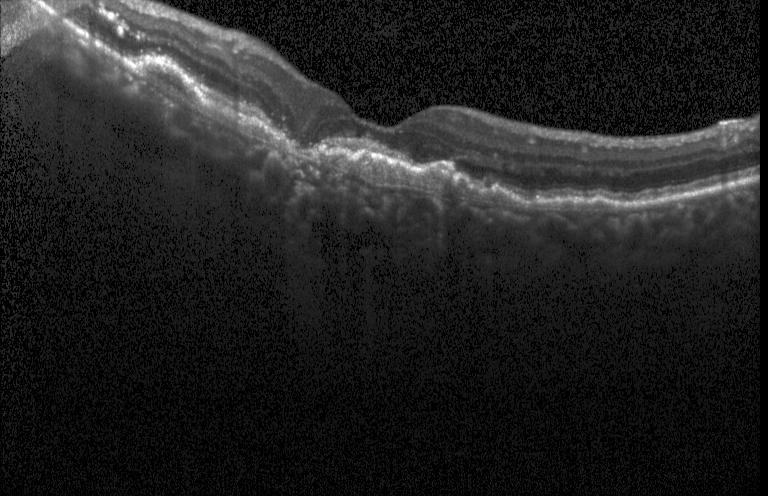
Diagnosis: a choroidal neovascular membrane.